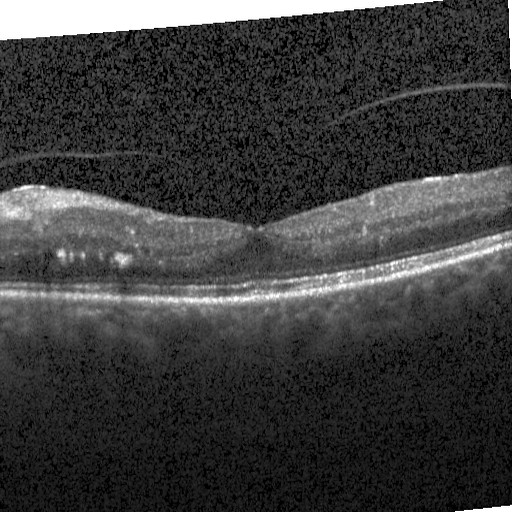 Acquired on a Heidelberg Spectralis; through the macula; spectral-domain optical coherence tomography; optical coherence tomography scan
Dx: diabetic macular edema.